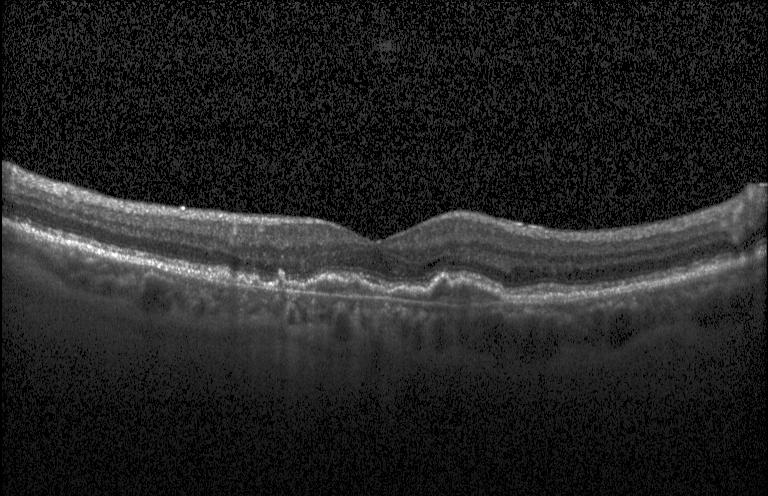

Dx: choroidal neovascularization.